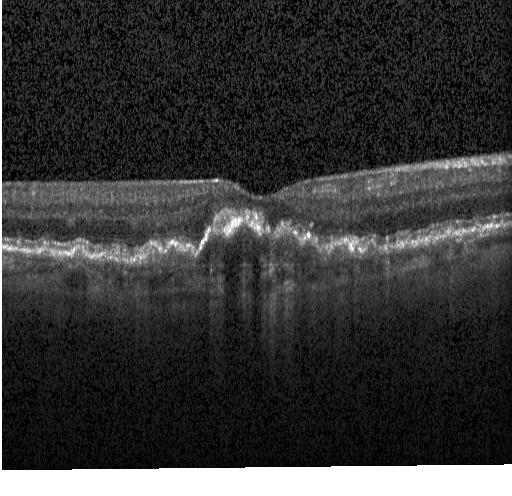

SD-OCT · centered on the fovea · Heidelberg Spectralis OCT system · optical coherence tomography scan — Finding: choroidal neovascularization.